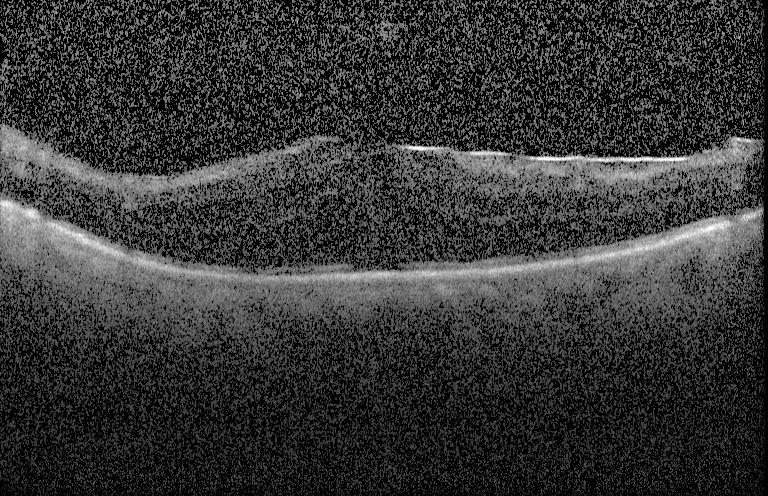

OCT B-scan showing DME.